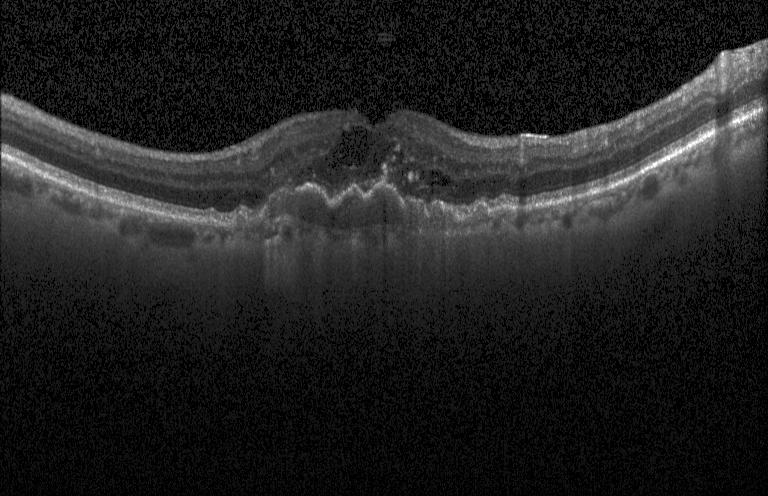

OCT finding: a choroidal neovascular membrane.